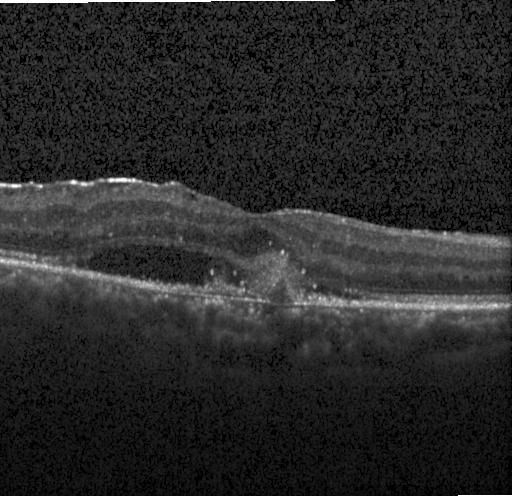

Instrument: Heidelberg Spectralis. OCT line scan. Impression: CNV.